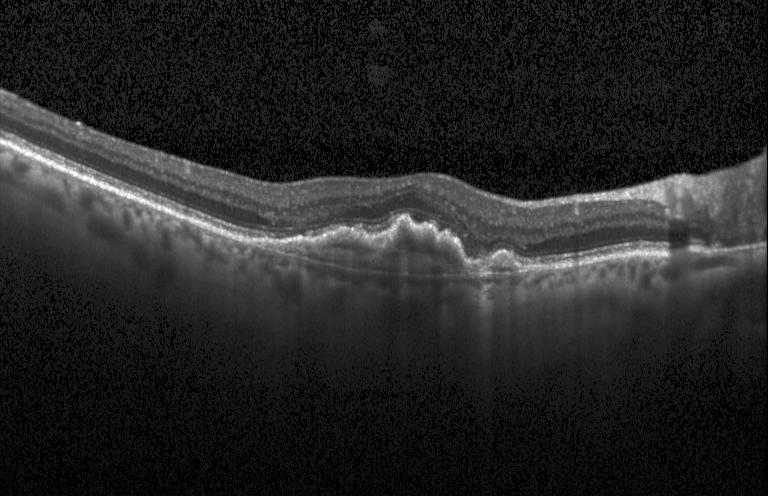

Acquired on a Heidelberg Spectralis · optical coherence tomography B-scan — Diagnosis: choroidal neovascularization.